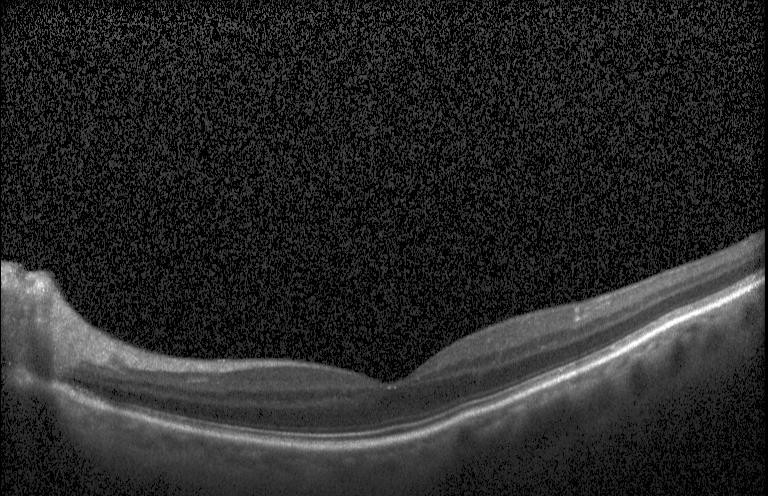

Optical coherence tomography B-scan.
The scan shows no evidence of choroidal neovascularization, diabetic macular edema, or drusen.